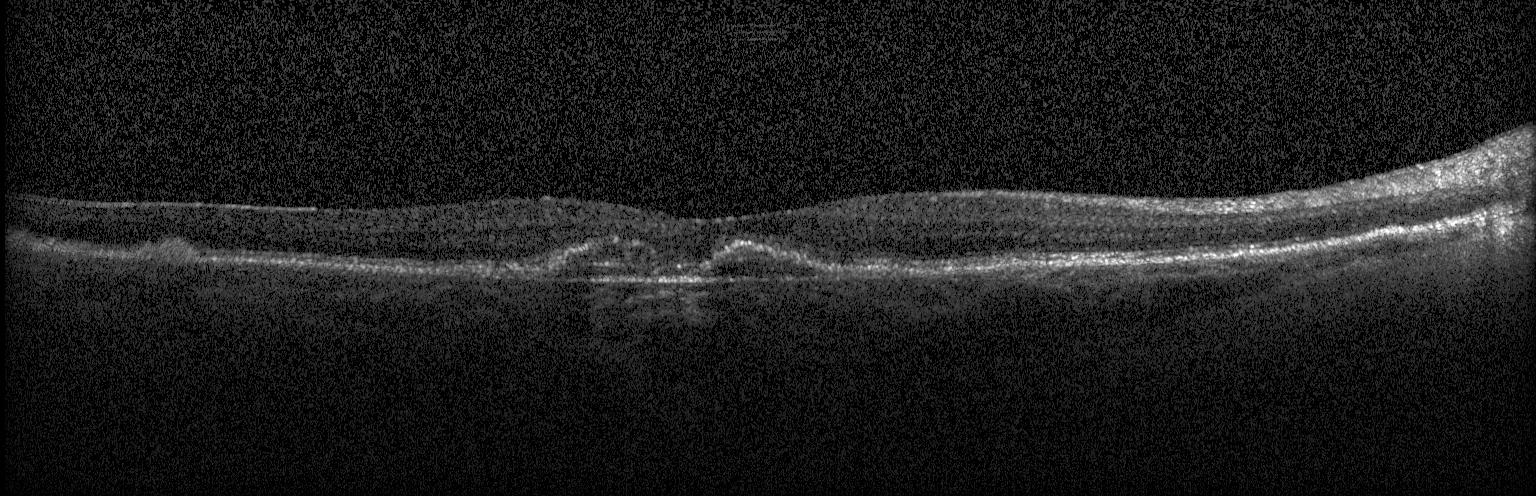

Diagnosis: a choroidal neovascular membrane.